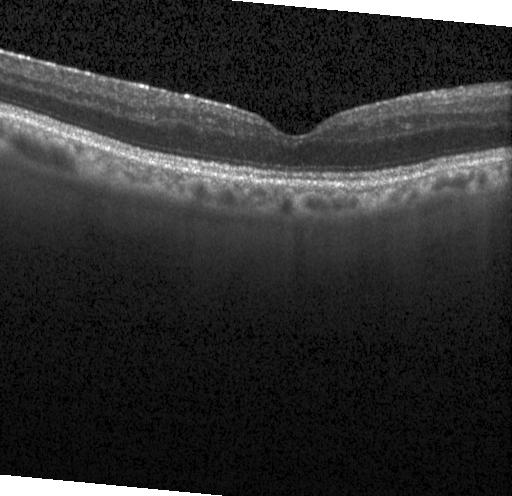
Assessment: no choroidal neovascularization, diabetic macular edema, or drusen.